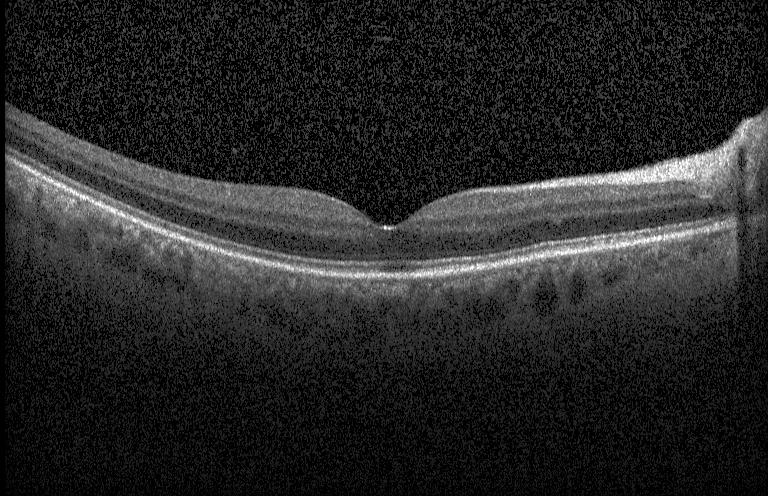
Optical coherence tomography scan. Assessment: no CNV, DME, or drusen.